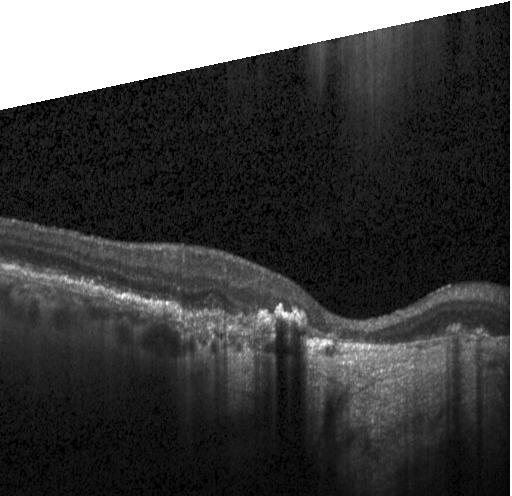

Horizontal scan through the fovea, optical coherence tomography scan, spectral-domain optical coherence tomography.
Finding: a choroidal neovascular membrane.